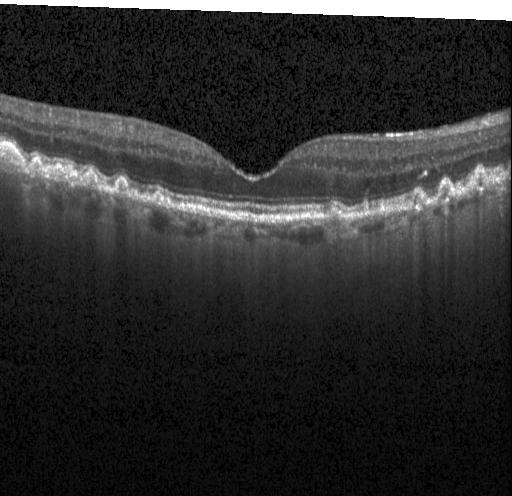
Dx: multiple drusen.